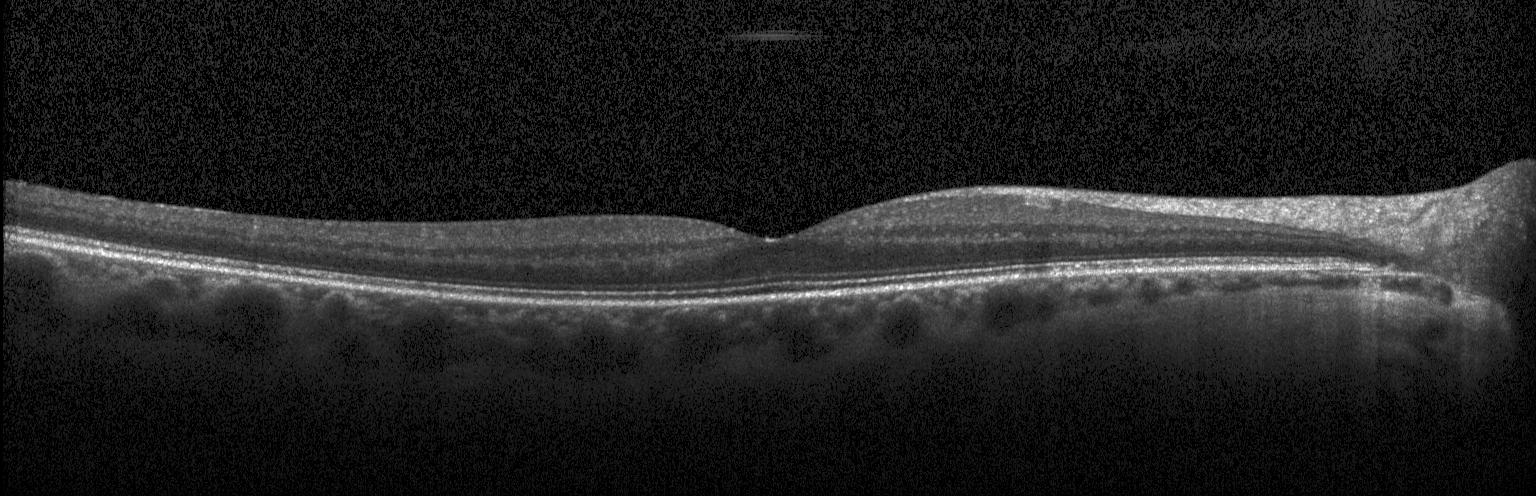 Assessment: no evidence of CNV, DME, or drusen.